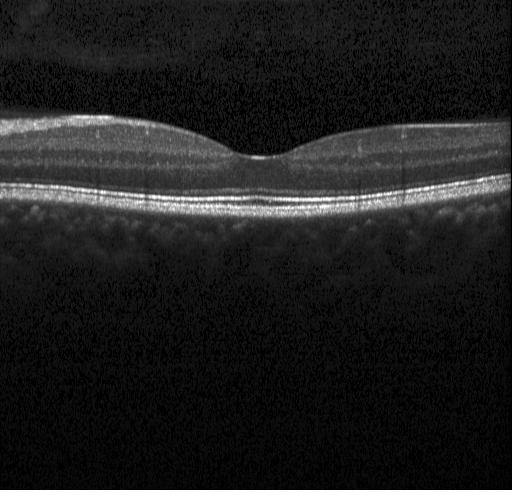
Assessment: neither choroidal neovascularization, diabetic macular edema, nor drusen.